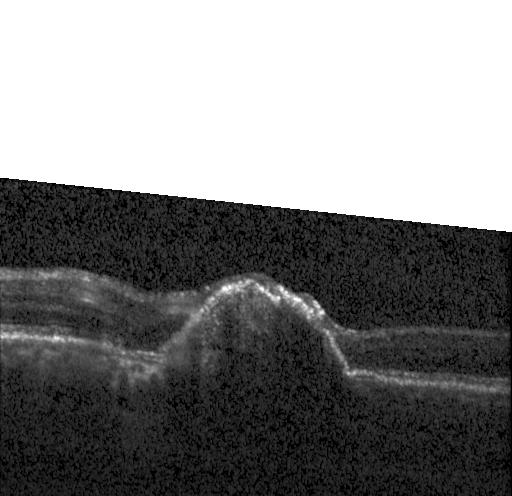
OCT line scan — Diagnosis: choroidal neovascularization (CNV).